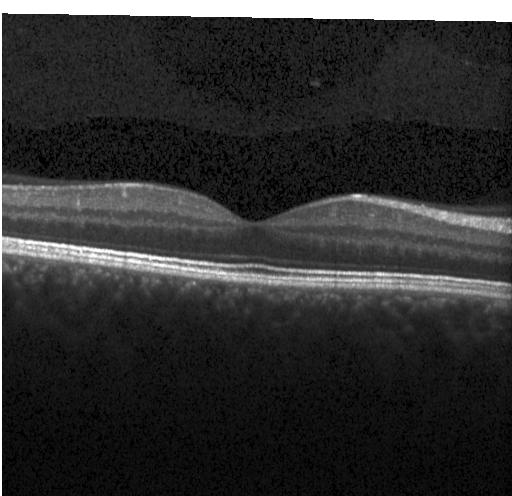

The scan shows neither CNV, DME, nor drusen.